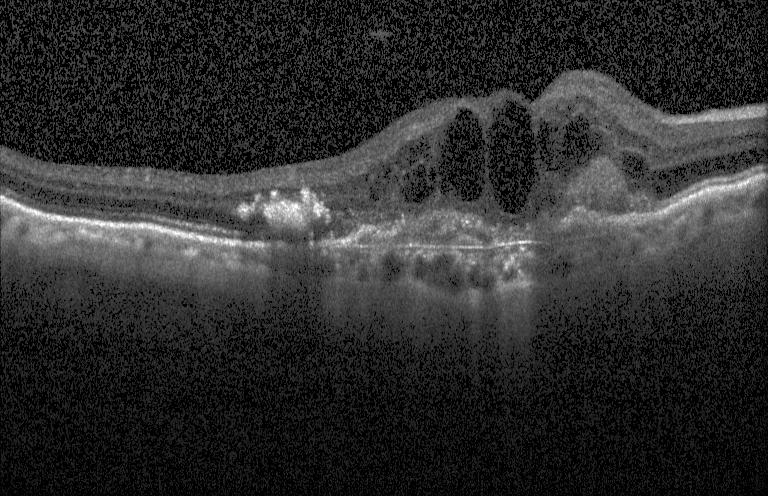 SD-OCT, retinal OCT B-scan, Heidelberg Spectralis, through the macula — Assessment: a choroidal neovascular membrane.